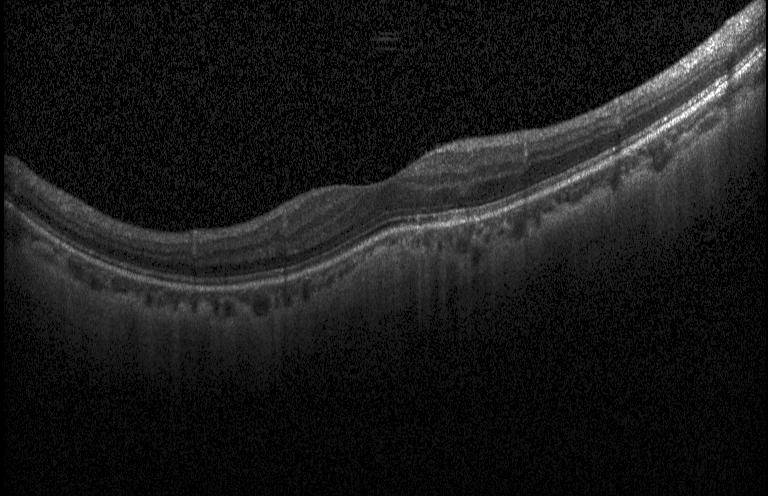

SD-OCT · optical coherence tomography scan · centered on the fovea · instrument: Heidelberg Spectralis.
Finding: no CNV, no DME, and no drusen.